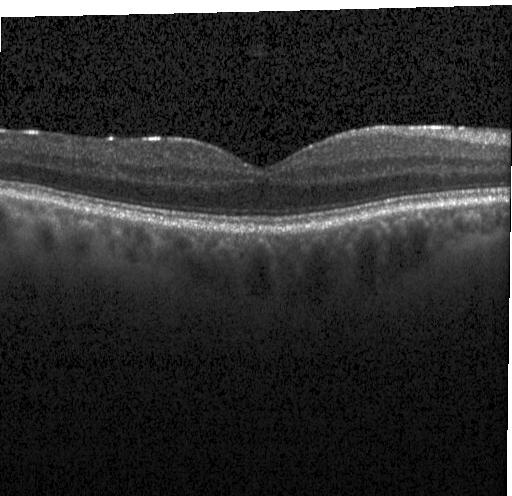
Retinal OCT cross-section, spectral-domain optical coherence tomography, through the macula, acquired on a Heidelberg Spectralis. Macular OCT: no evidence of CNV, DME, or drusen.